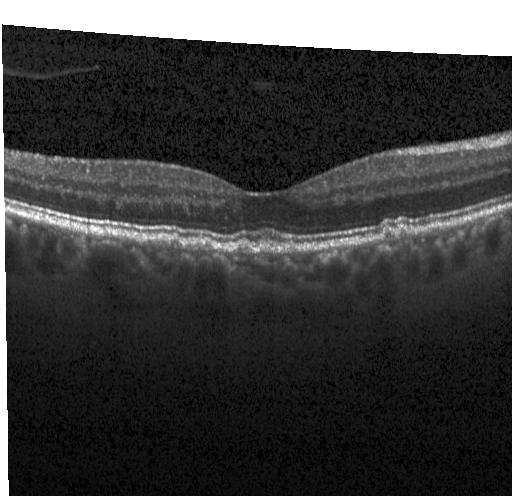 Instrument: Heidelberg Spectralis. Optical coherence tomography B-scan. Macular scan. Finding: drusen.